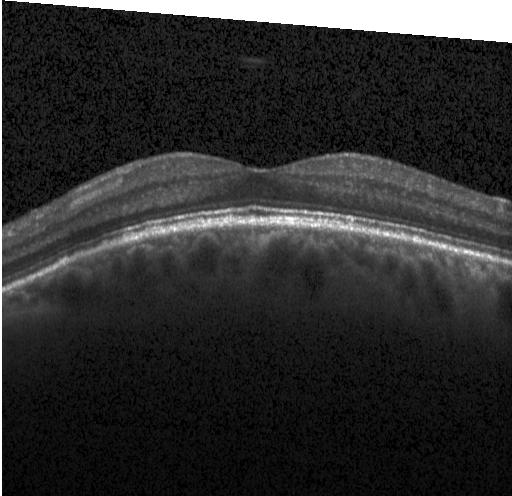
Retinal OCT cross-section, horizontal scan through the fovea. Diagnosis: neither CNV, DME, nor drusen.